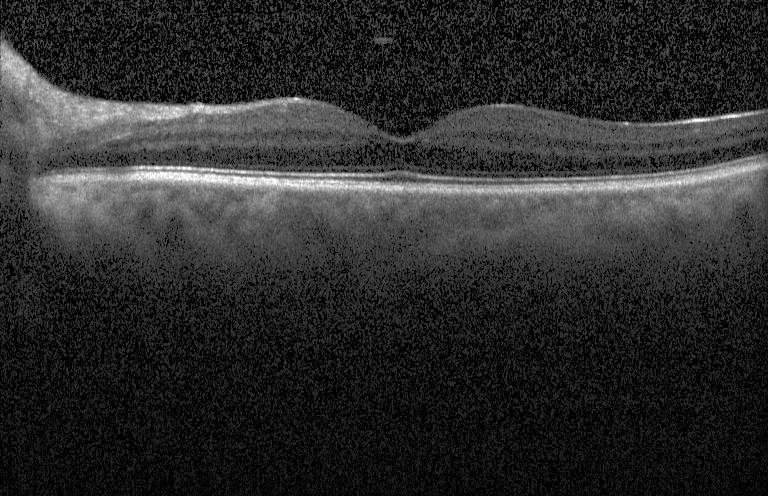

Optical coherence tomography B-scan. Fovea-centered. Acquired on a Heidelberg Spectralis. Spectral-domain optical coherence tomography. No choroidal neovascularization, diabetic macular edema, or drusen.